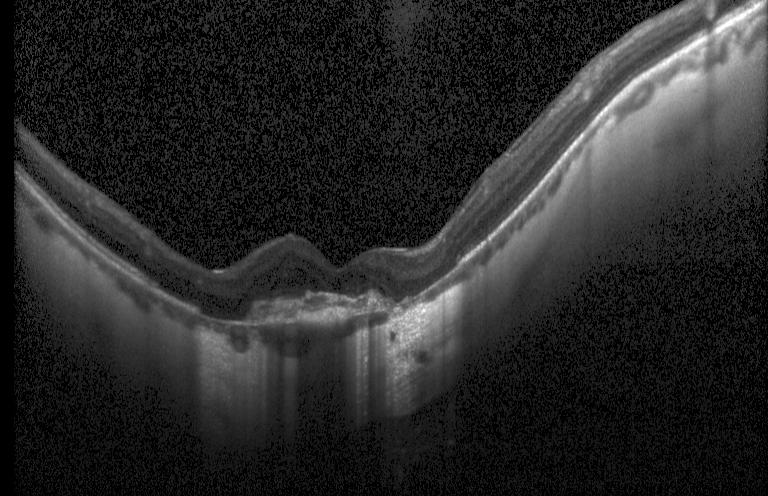 OCT finding: a choroidal neovascular membrane.